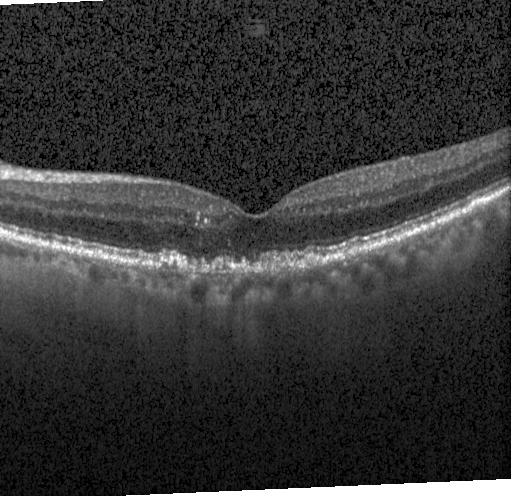

Retinal OCT cross-section showing drusen.